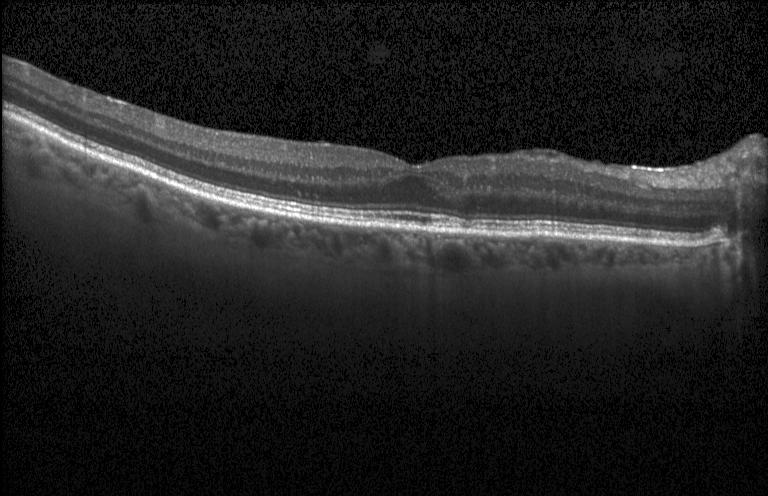 Spectral-domain optical coherence tomography. OCT B-scan.
Impression: no choroidal neovascularization, no diabetic macular edema, and no drusen.